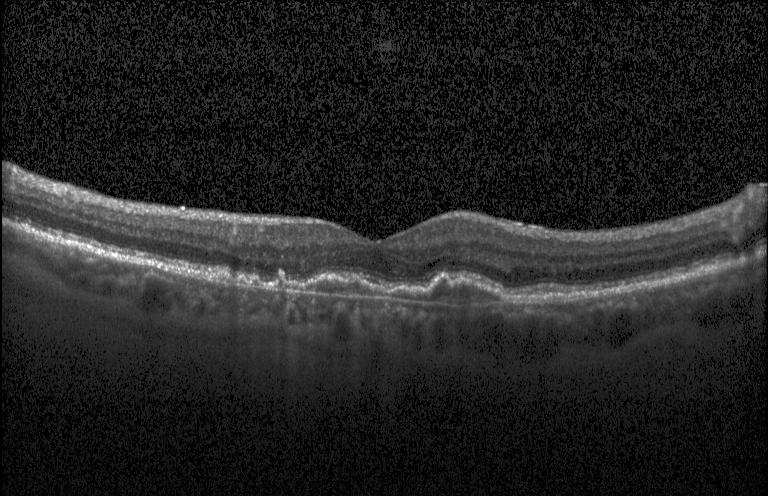
Dx: CNV.